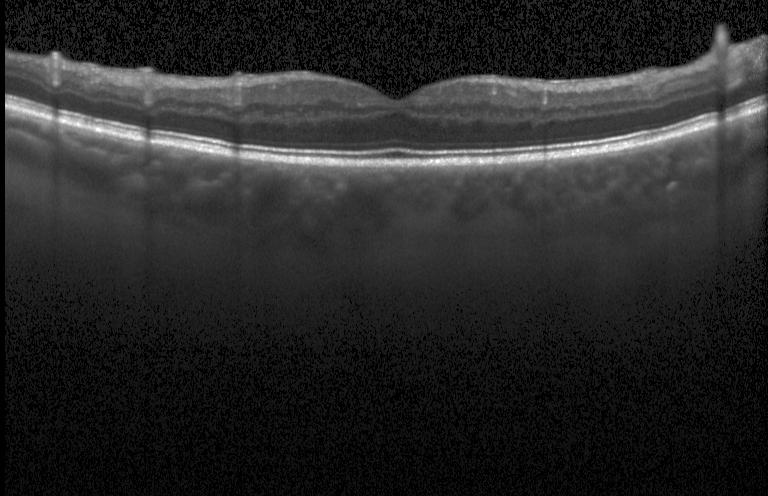

Retinal OCT cross-section showing no CNV, no DME, and no drusen.